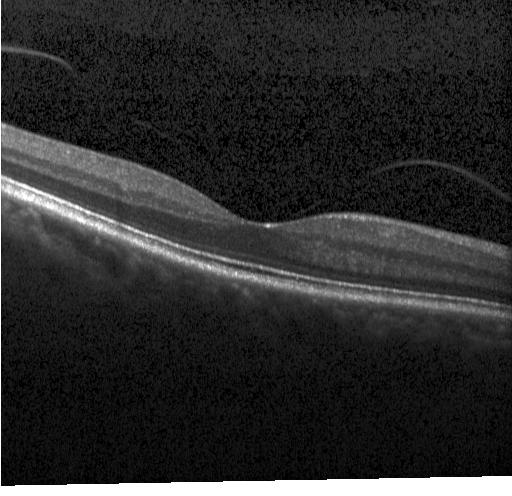 This B-scan demonstrates no evidence of CNV, DME, or drusen.